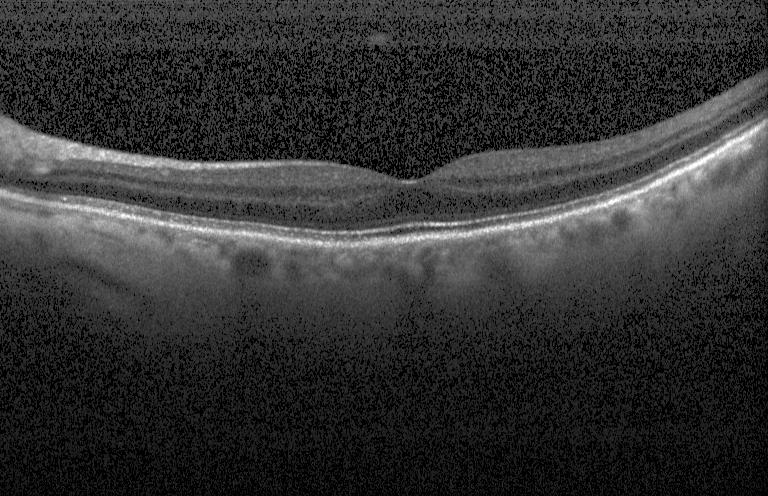
Impression: no choroidal neovascularization, no diabetic macular edema, and no drusen.